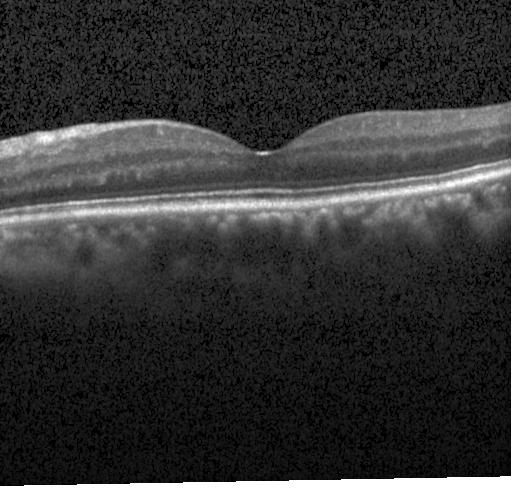 Spectral-domain OCT. Retinal OCT B-scan.
OCT finding: neither choroidal neovascularization, diabetic macular edema, nor drusen.